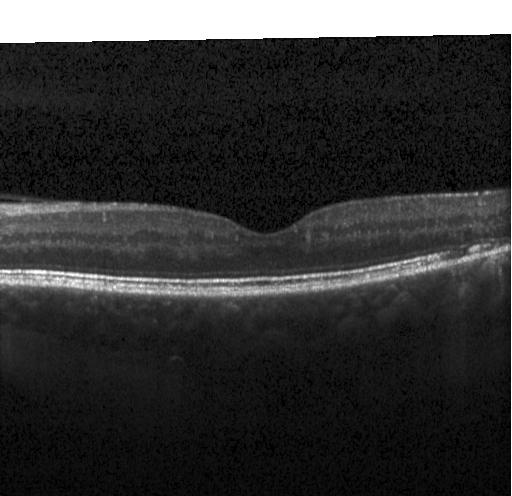
Macular scan. Optical coherence tomography scan. Assessment: no CNV, DME, or drusen.